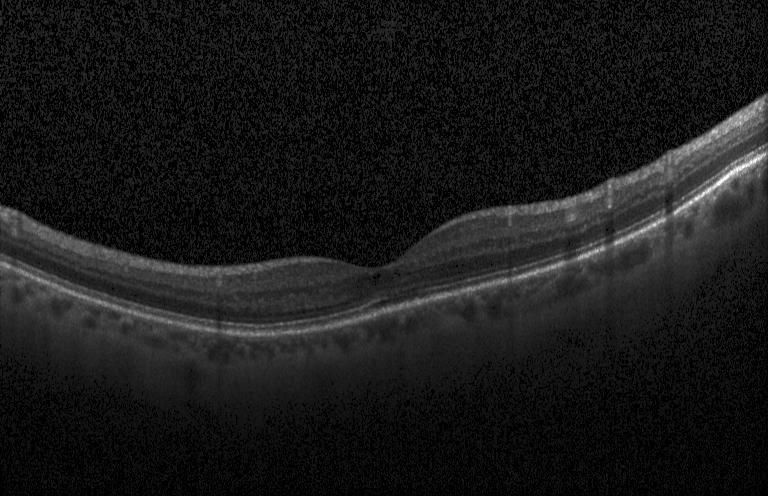
Optical coherence tomography B-scan, spectral-domain optical coherence tomography, fovea-centered — This B-scan demonstrates no CNV, no DME, and no drusen.